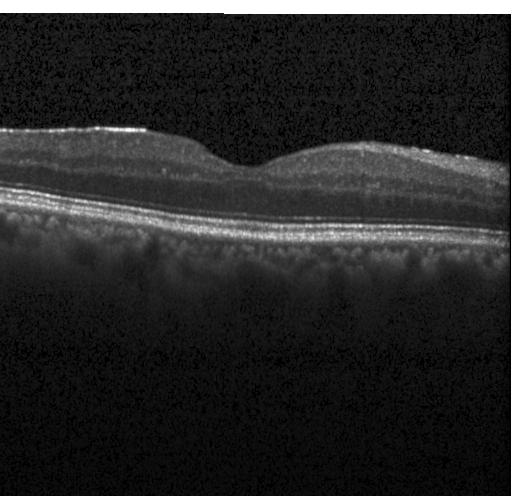 Retinal OCT B-scan
Dx: neither choroidal neovascularization, diabetic macular edema, nor drusen.